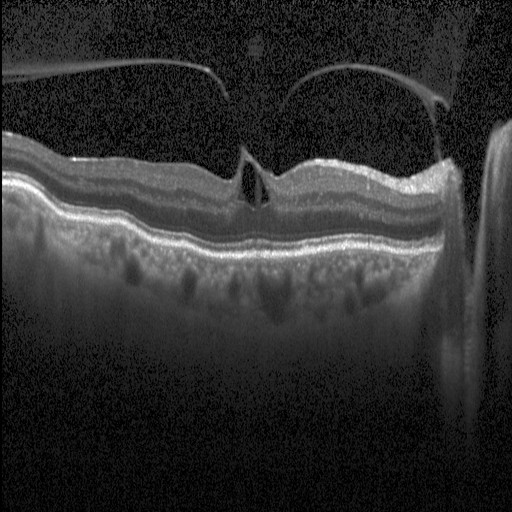

Instrument: Heidelberg Spectralis · optical coherence tomography B-scan — OCT finding: DME.